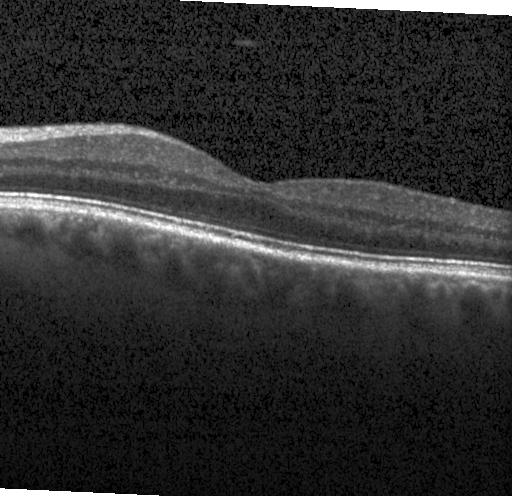

Heidelberg Spectralis OCT system · retinal OCT B-scan.
Finding: no CNV, DME, or drusen.